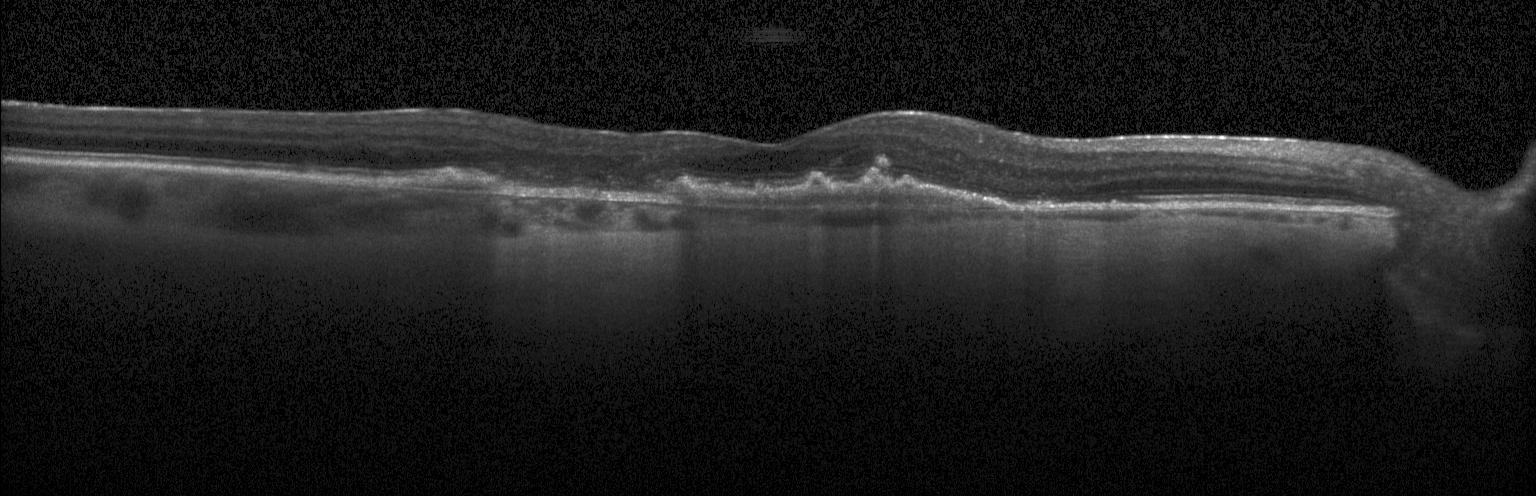

Retinal OCT cross-section. OCT finding: choroidal neovascularization (CNV).